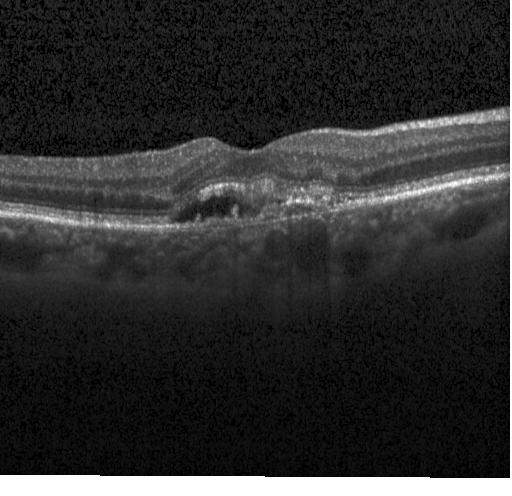 Instrument: Heidelberg Spectralis; spectral-domain OCT; centered on the fovea; retinal OCT B-scan. Impression: a choroidal neovascular membrane.